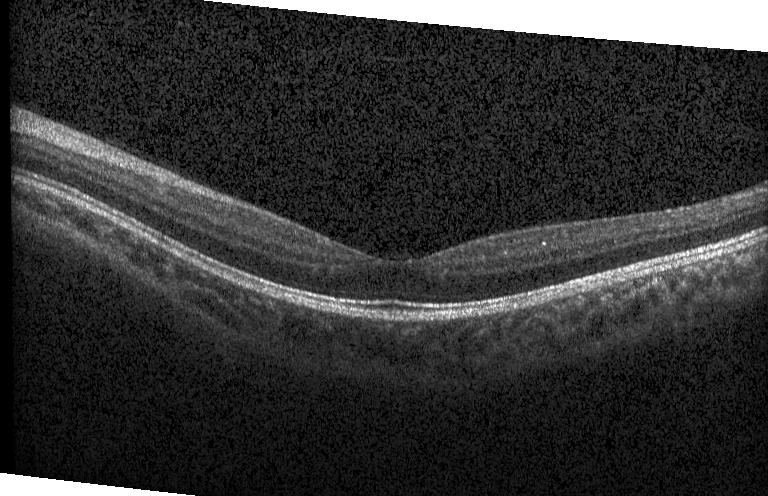
Finding: no choroidal neovascularization, diabetic macular edema, or drusen.